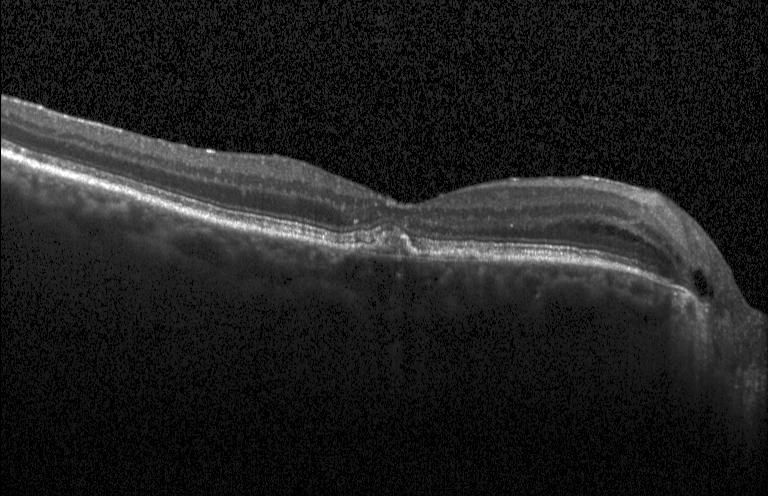

Retinal OCT cross-section · spectral-domain optical coherence tomography · fovea-centered · acquired on a Heidelberg Spectralis — Diagnosis: a choroidal neovascular membrane.